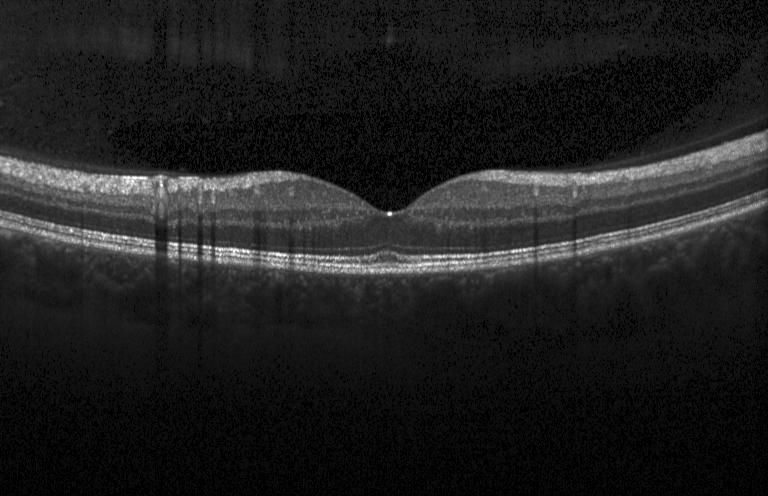
Optical coherence tomography scan · macular scan · SD-OCT · instrument: Heidelberg Spectralis. Finding: no evidence of choroidal neovascularization, diabetic macular edema, or drusen.